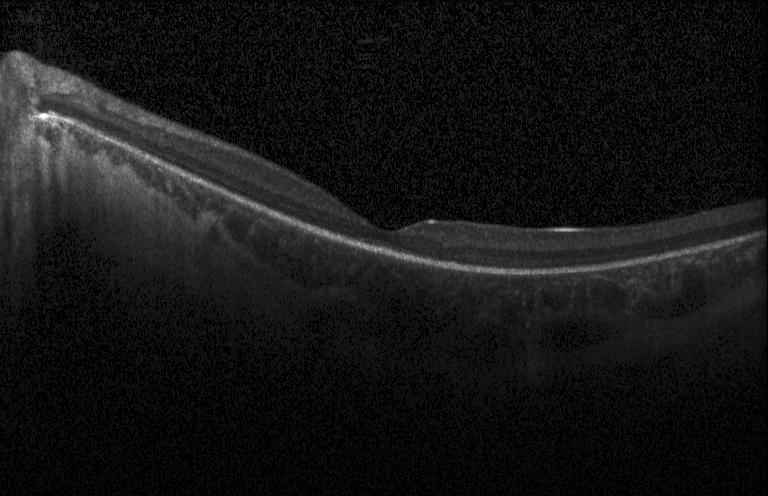 Dx: neither CNV, DME, nor drusen.